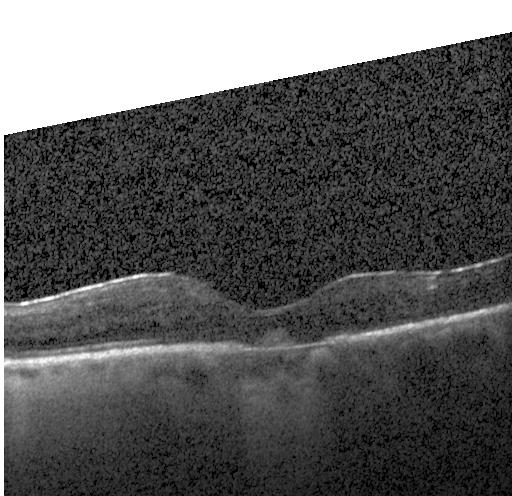 Diagnosis: a choroidal neovascular membrane.